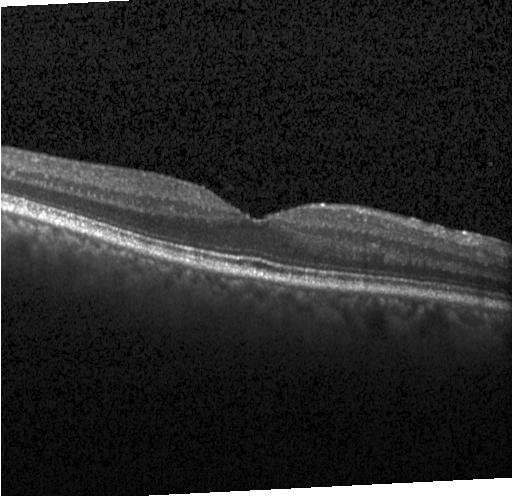
No choroidal neovascularization, diabetic macular edema, or drusen.